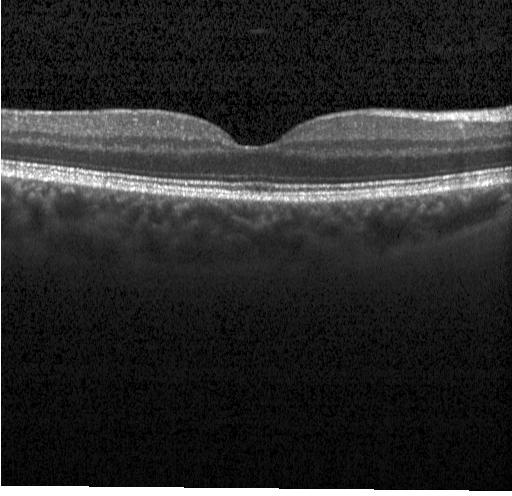 Finding: neither CNV, DME, nor drusen.